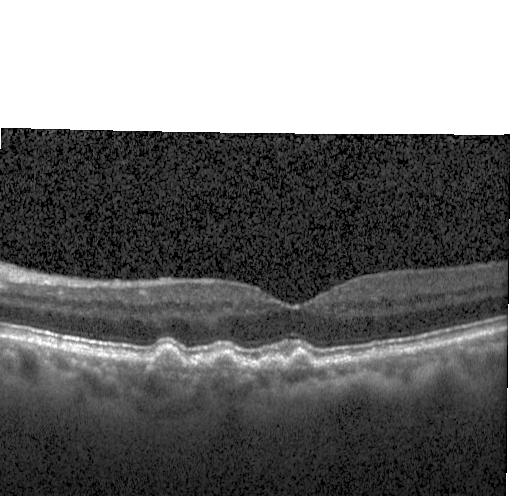 OCT B-scan. Instrument: Heidelberg Spectralis. Fovea-centered. Spectral-domain OCT — This B-scan demonstrates multiple drusen.